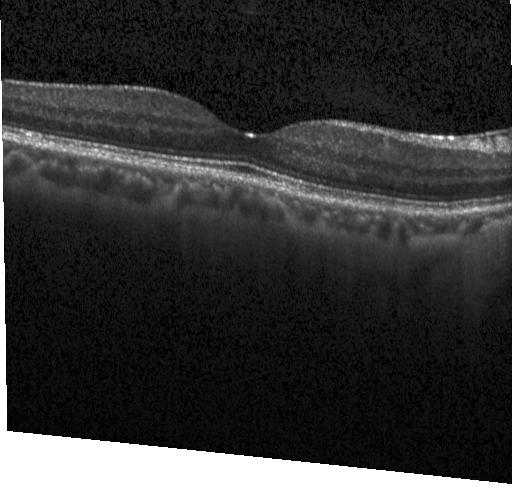
Heidelberg Spectralis OCT system. Optical coherence tomography scan. Finding: neither choroidal neovascularization, diabetic macular edema, nor drusen.